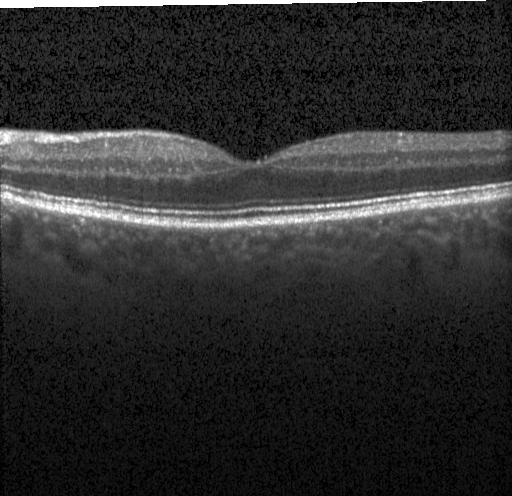 OCT B-scan showing neither choroidal neovascularization, diabetic macular edema, nor drusen.